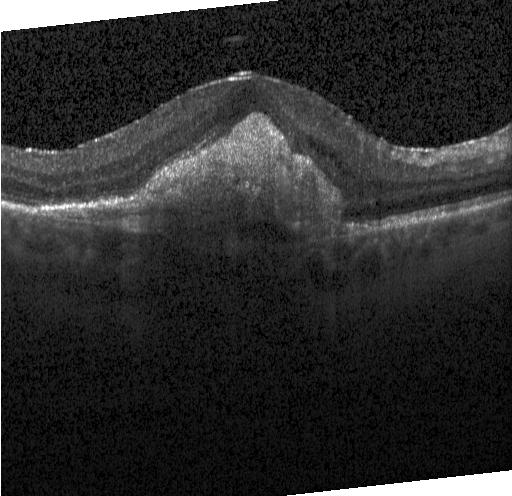

Dx: a choroidal neovascular membrane.